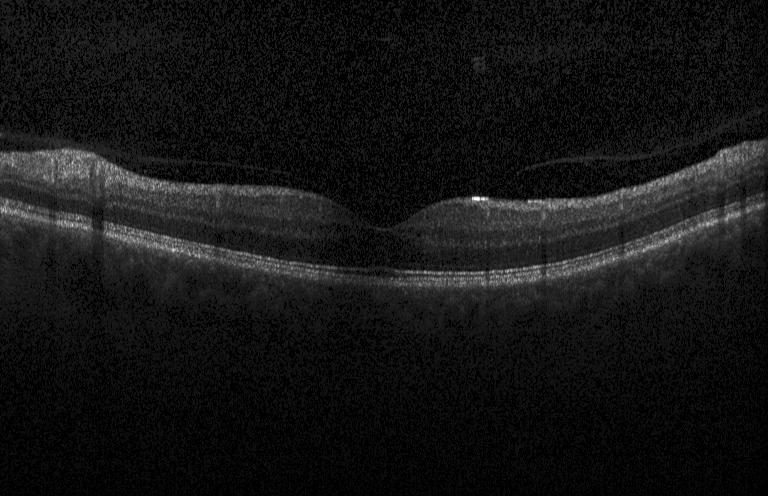 Diagnosis: no evidence of CNV, DME, or drusen.